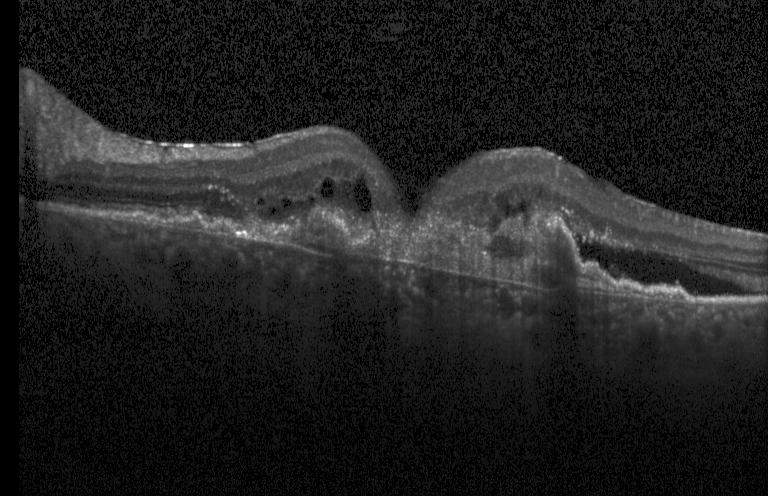 Retinal OCT cross-section. Diagnosis: a choroidal neovascular membrane.